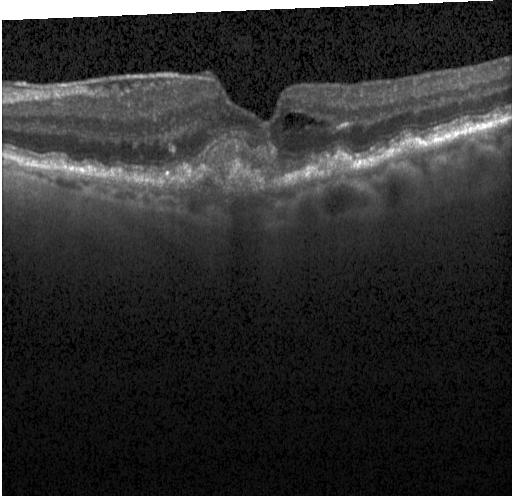

OCT B-scan showing choroidal neovascularization.